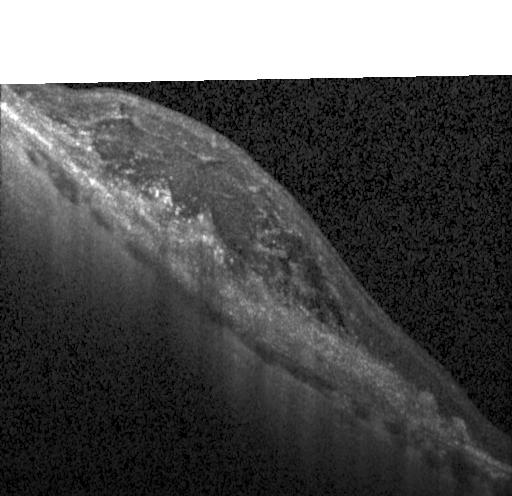
OCT B-scan, SD-OCT, horizontal scan through the fovea — Diagnosis: a choroidal neovascular membrane.